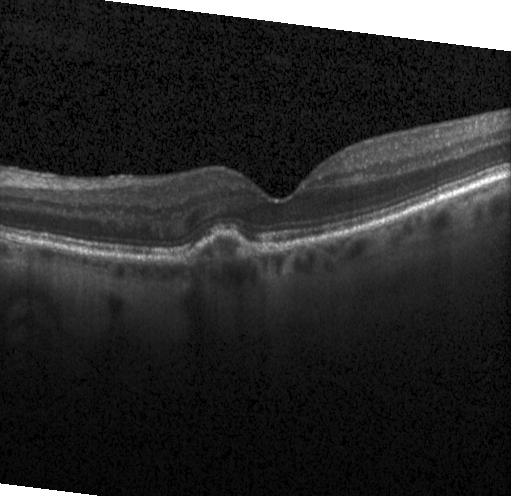
Optical coherence tomography B-scan · acquired on a Heidelberg Spectralis. Diagnosis: choroidal neovascularization (CNV).